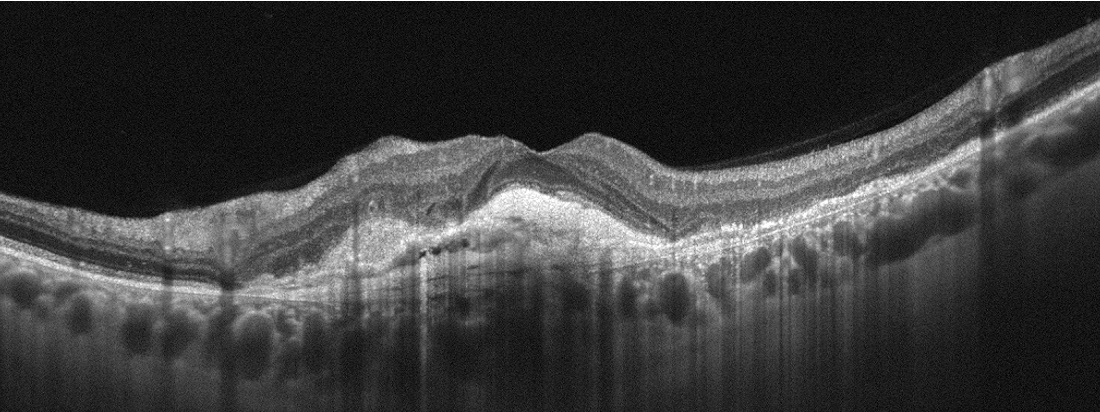
Through the macula, OCT B-scan. The scan shows AMD.